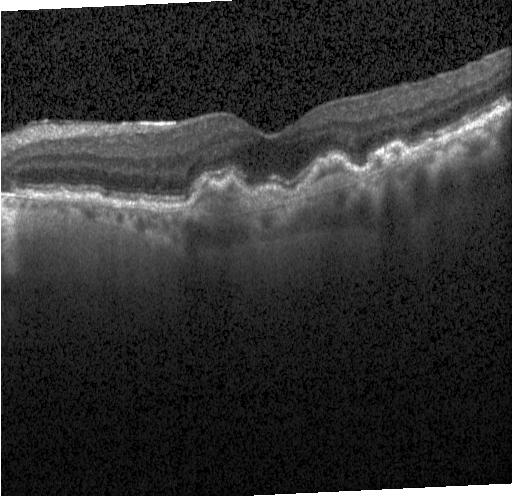 Fovea-centered · retinal OCT cross-section — The scan shows CNV.